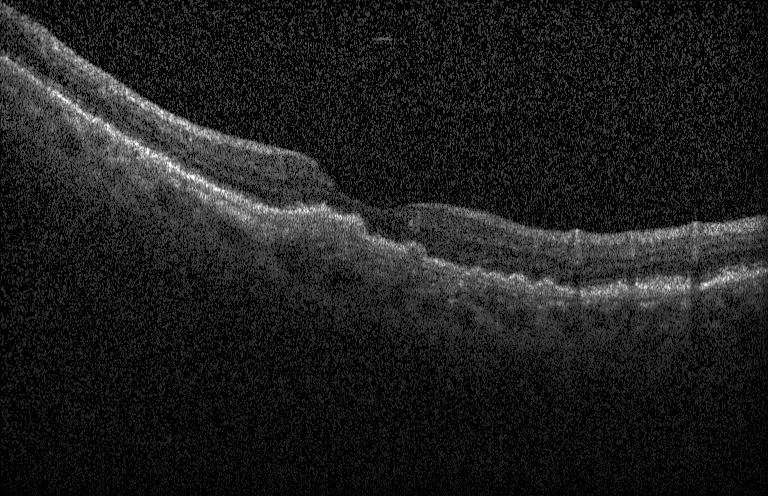 Finding: choroidal neovascularization.